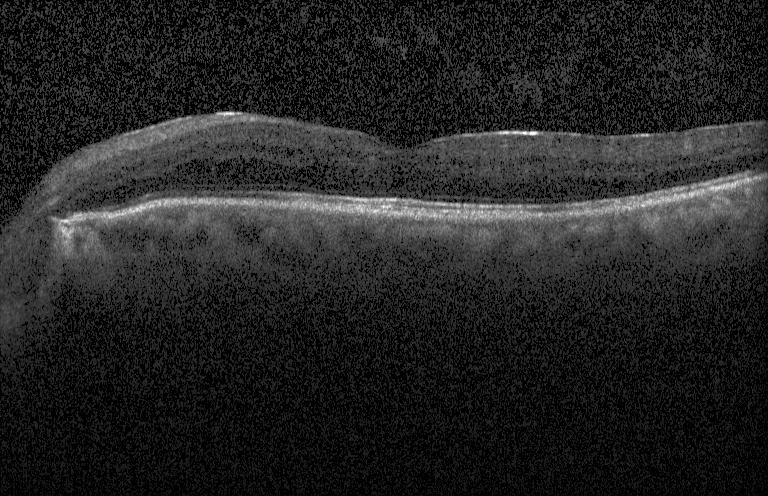
Macular OCT: no choroidal neovascularization, no diabetic macular edema, and no drusen.